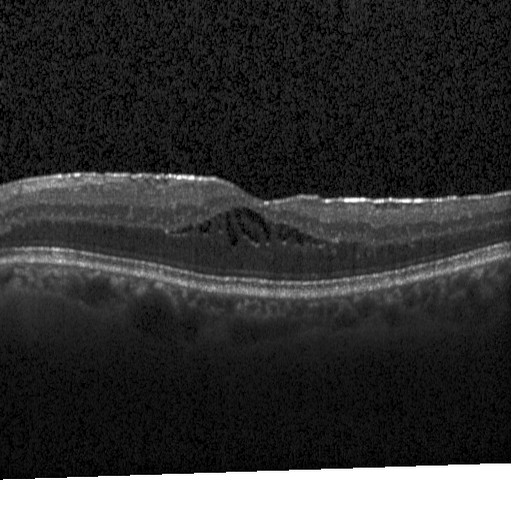 Heidelberg Spectralis OCT system · through the macula · OCT B-scan.
Diabetic macular edema (DME).